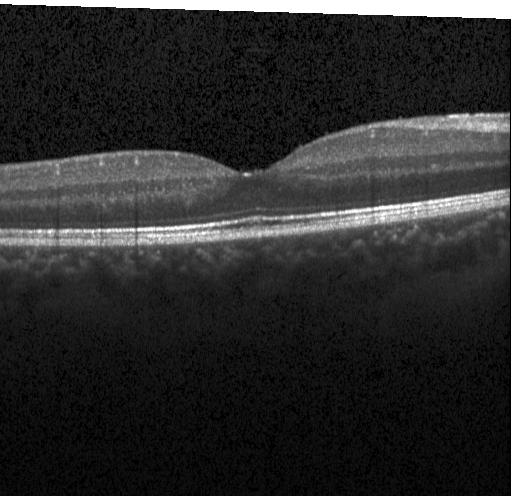
Retinal OCT cross-section, acquired on a Heidelberg Spectralis
Impression: no CNV, no DME, and no drusen.